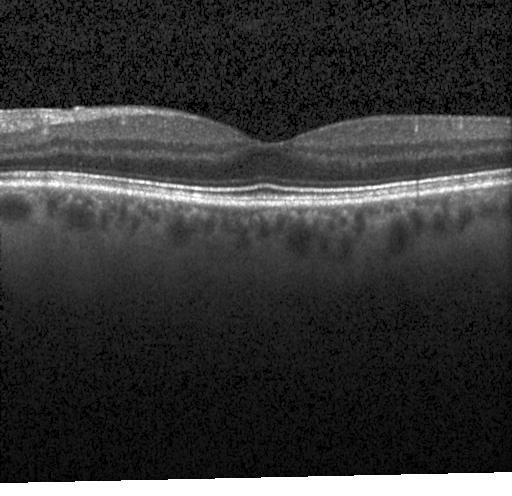 OCT scan showing neither CNV, DME, nor drusen.